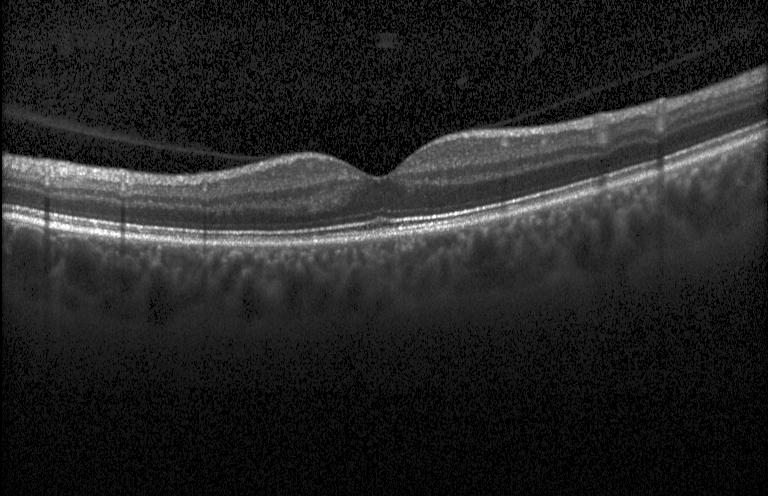
OCT finding: no choroidal neovascularization, diabetic macular edema, or drusen.